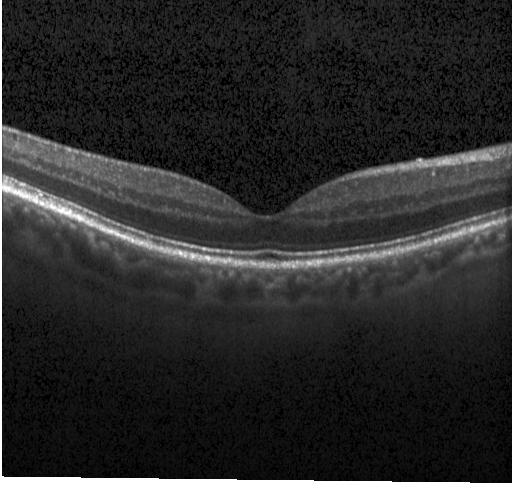

OCT line scan. Heidelberg Spectralis OCT system. Spectral-domain optical coherence tomography. Macular OCT: no choroidal neovascularization, no diabetic macular edema, and no drusen.